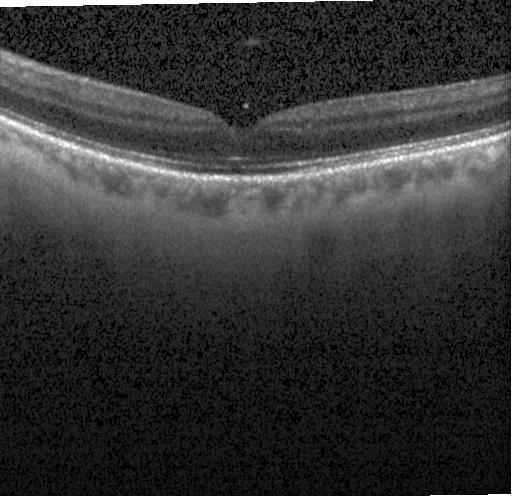
Dx: no choroidal neovascularization, diabetic macular edema, or drusen.